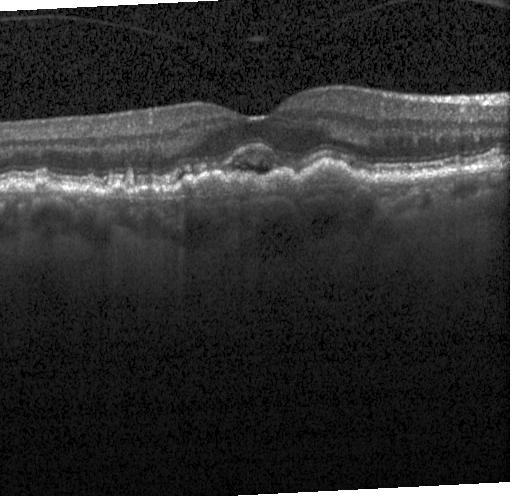

Dx: a choroidal neovascular membrane.